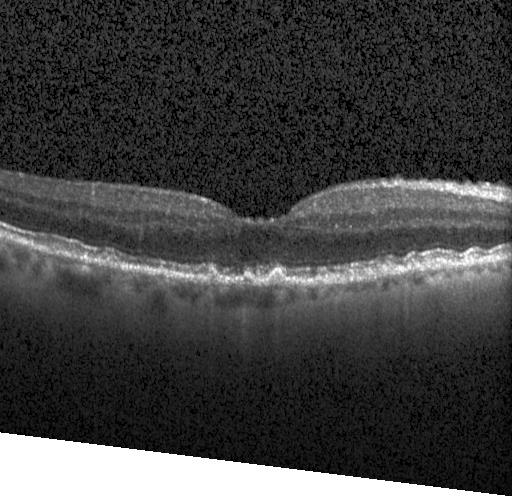

OCT line scan — The scan shows multiple drusen.